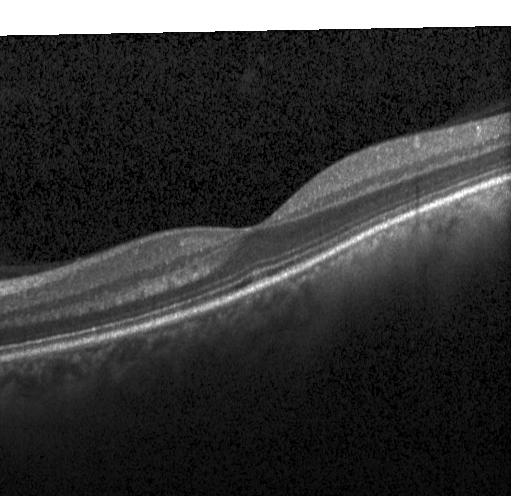 Impression: no evidence of choroidal neovascularization, diabetic macular edema, or drusen.